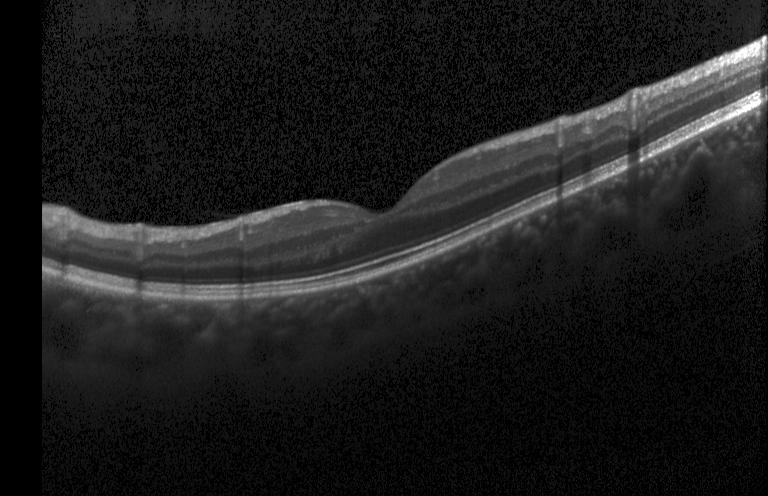

Impression: no choroidal neovascularization, diabetic macular edema, or drusen.